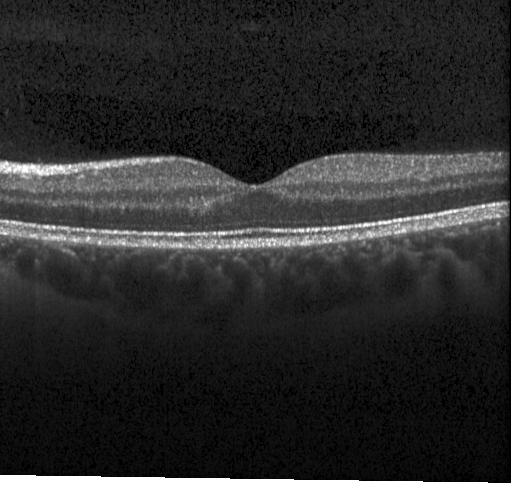
Macular scan. OCT line scan. Instrument: Heidelberg Spectralis.
Dx: no CNV, no DME, and no drusen.